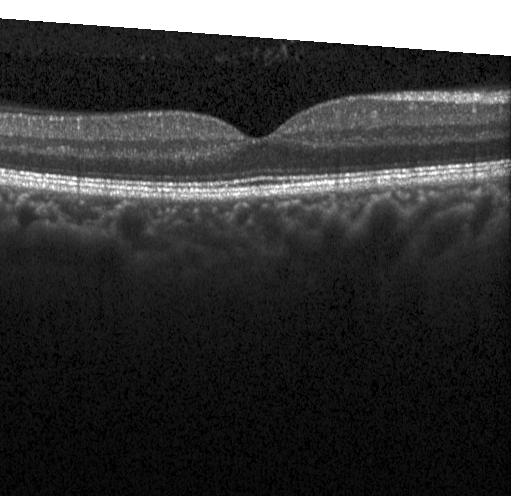

Macular OCT demonstrating neither choroidal neovascularization, diabetic macular edema, nor drusen.